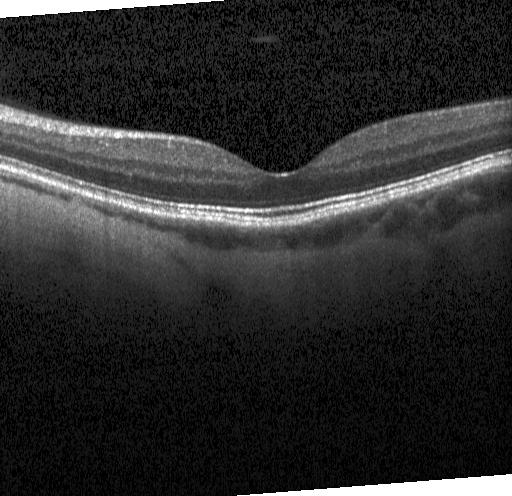
Optical coherence tomography B-scan. Finding: no evidence of CNV, DME, or drusen.